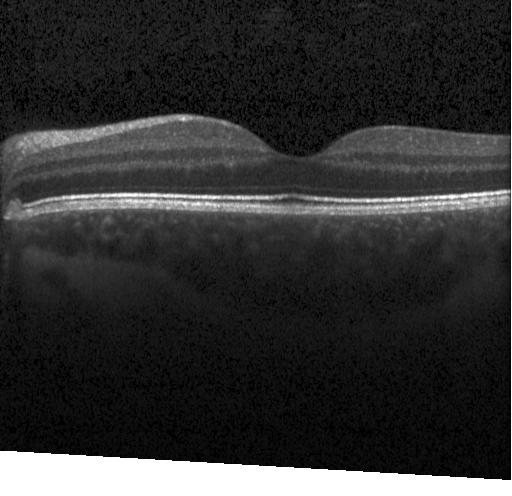

Optical coherence tomography scan, spectral-domain optical coherence tomography, fovea-centered.
Assessment: neither choroidal neovascularization, diabetic macular edema, nor drusen.